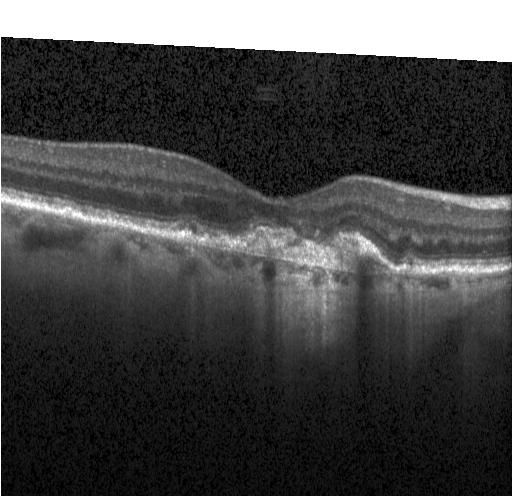

Assessment: a choroidal neovascular membrane.